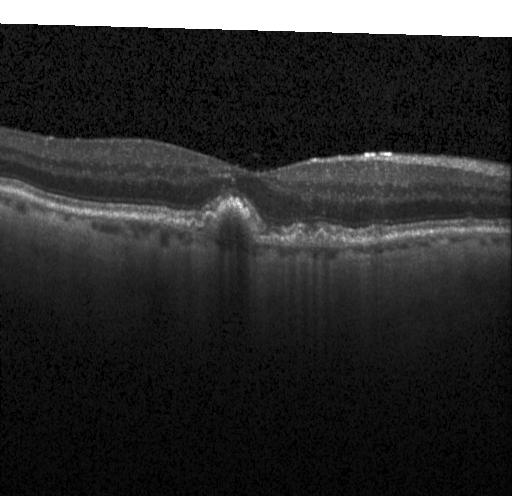

Optical coherence tomography B-scan, macular scan
Finding: multiple drusen.